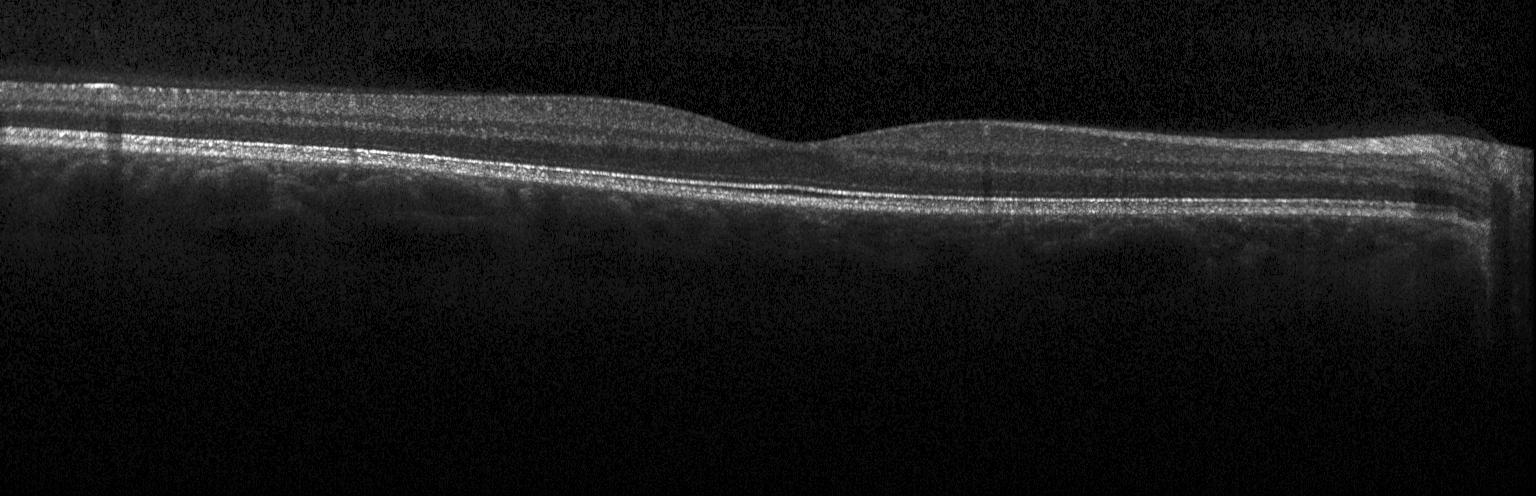
Optical coherence tomography B-scan
Diagnosis: neither choroidal neovascularization, diabetic macular edema, nor drusen.